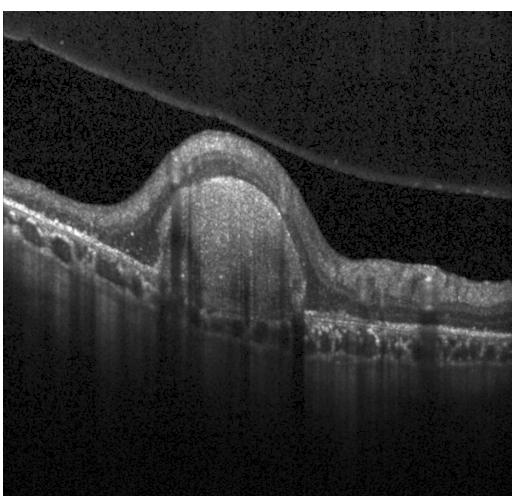 OCT B-scan — Assessment: a choroidal neovascular membrane.